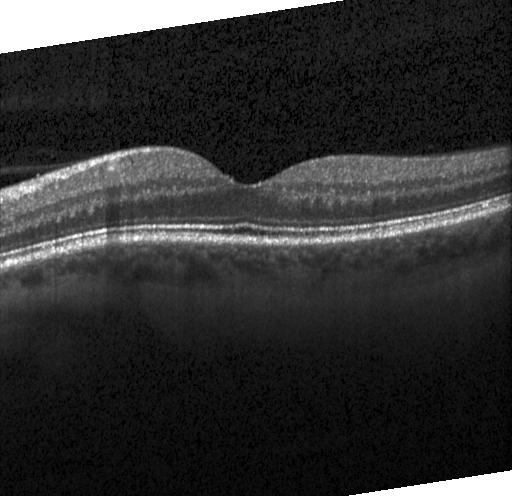

Horizontal scan through the fovea, spectral-domain optical coherence tomography, optical coherence tomography B-scan
This B-scan demonstrates neither choroidal neovascularization, diabetic macular edema, nor drusen.